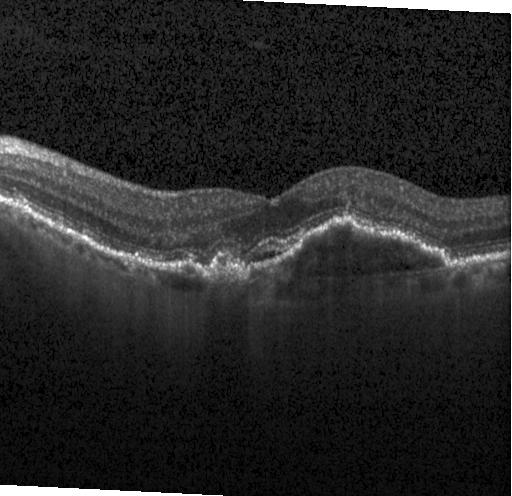
OCT line scan; spectral-domain OCT. Finding: CNV.